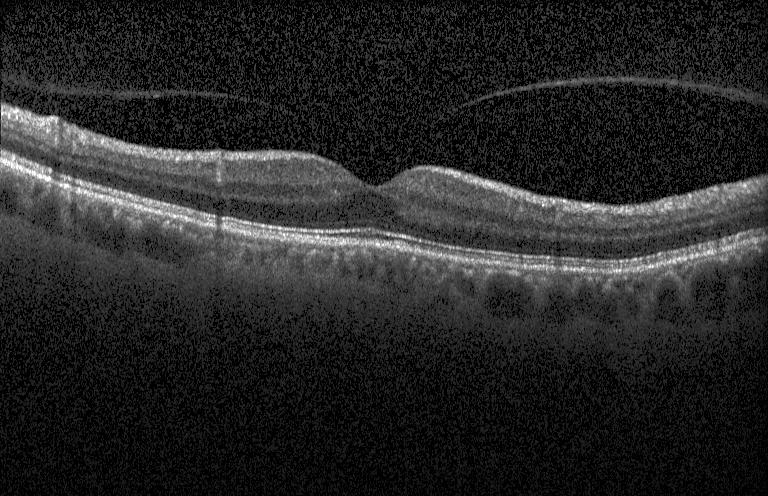 Finding: no evidence of choroidal neovascularization, diabetic macular edema, or drusen.